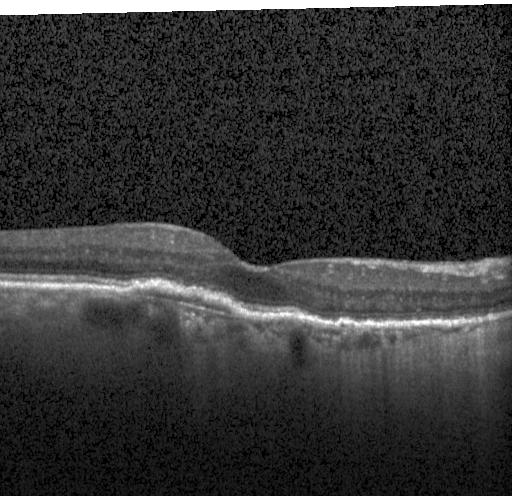 Spectral-domain OCT · OCT B-scan.
Dx: a choroidal neovascular membrane.